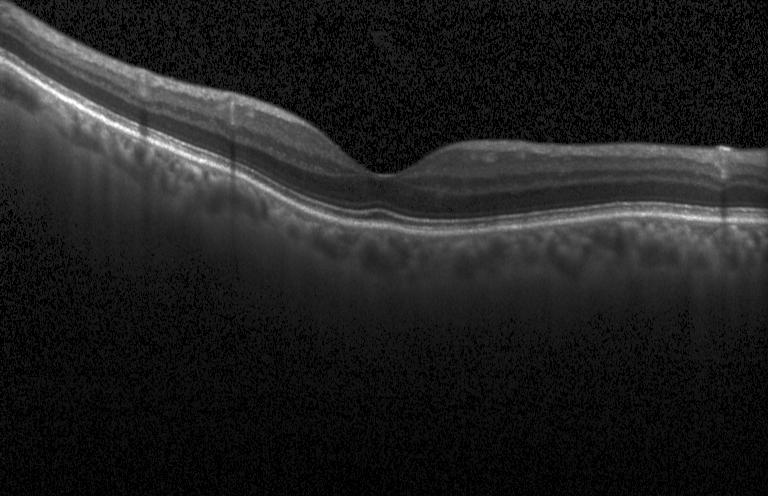
Optical coherence tomography B-scan. Diagnosis: no choroidal neovascularization, diabetic macular edema, or drusen.